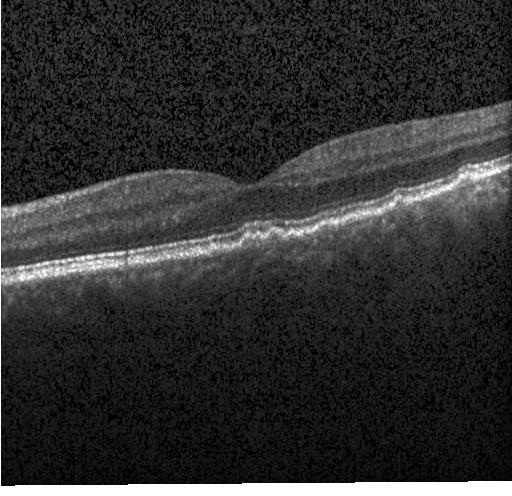

Heidelberg Spectralis OCT system, fovea-centered, OCT B-scan.
Macular OCT: multiple drusen.